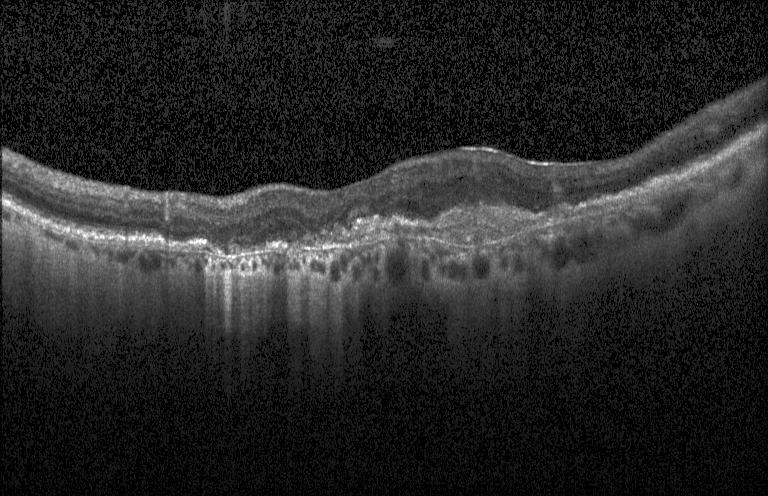 Macular OCT: choroidal neovascularization.